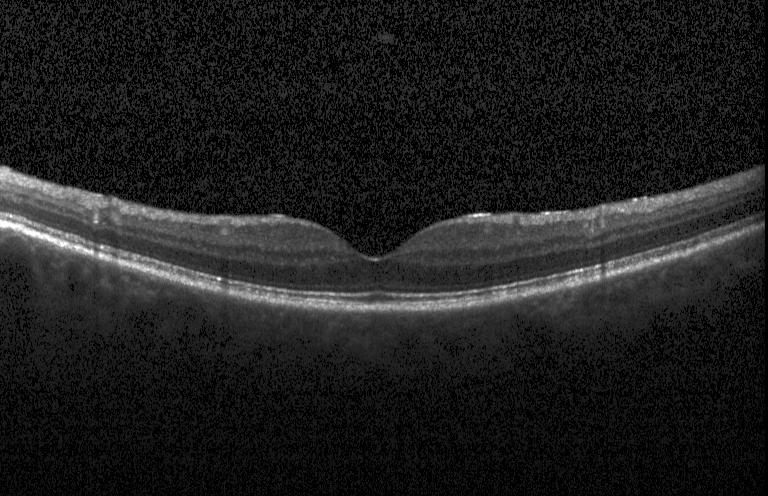

Impression: no choroidal neovascularization, diabetic macular edema, or drusen.